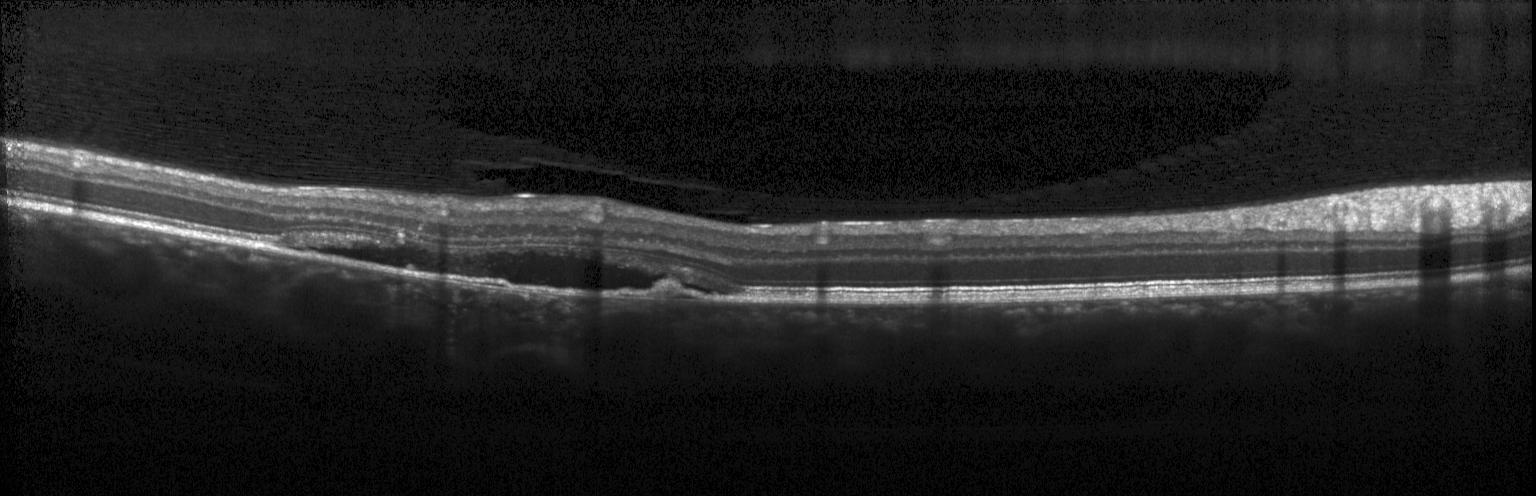
OCT B-scan; spectral-domain optical coherence tomography; Heidelberg Spectralis
Diagnosis: CNV.